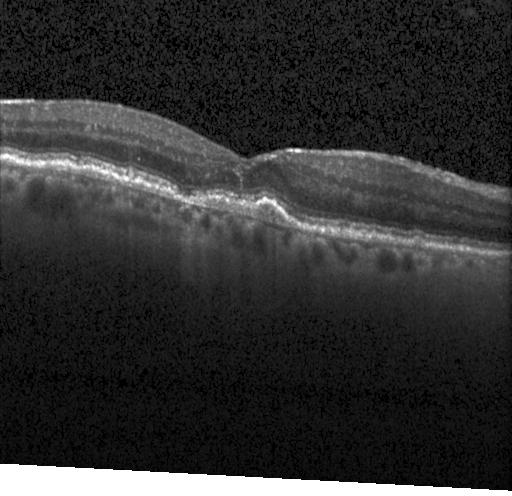
SD-OCT · OCT B-scan · acquired on a Heidelberg Spectralis — Impression: choroidal neovascularization.